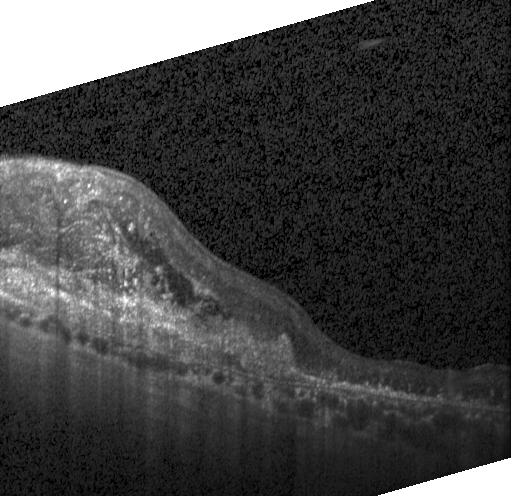

Impression: choroidal neovascularization (CNV).